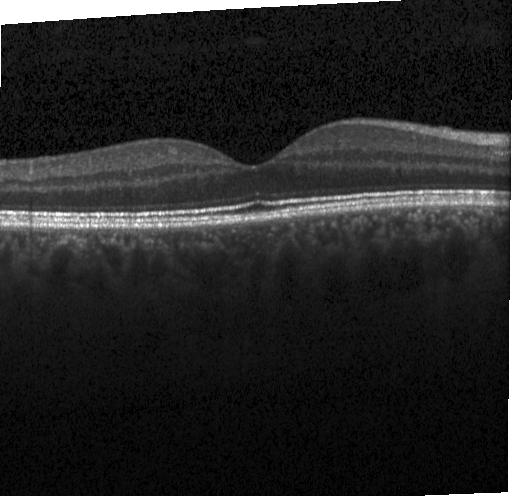 Dx: no evidence of choroidal neovascularization, diabetic macular edema, or drusen.